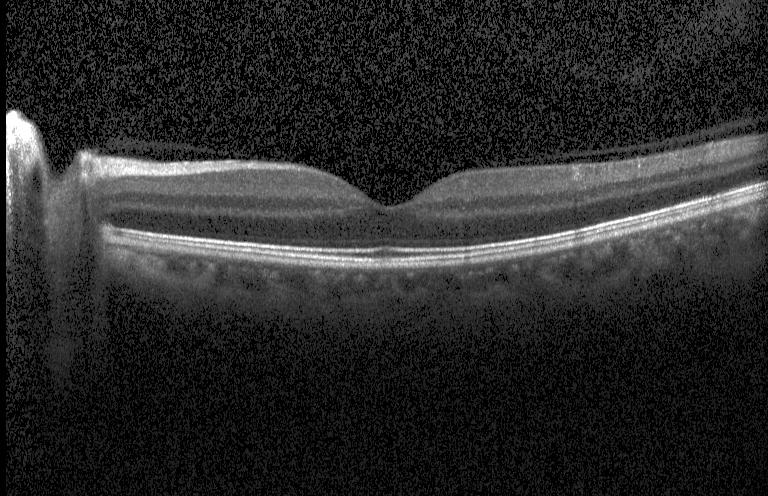 Acquired on a Heidelberg Spectralis, retinal OCT B-scan, centered on the fovea.
Assessment: no evidence of choroidal neovascularization, diabetic macular edema, or drusen.